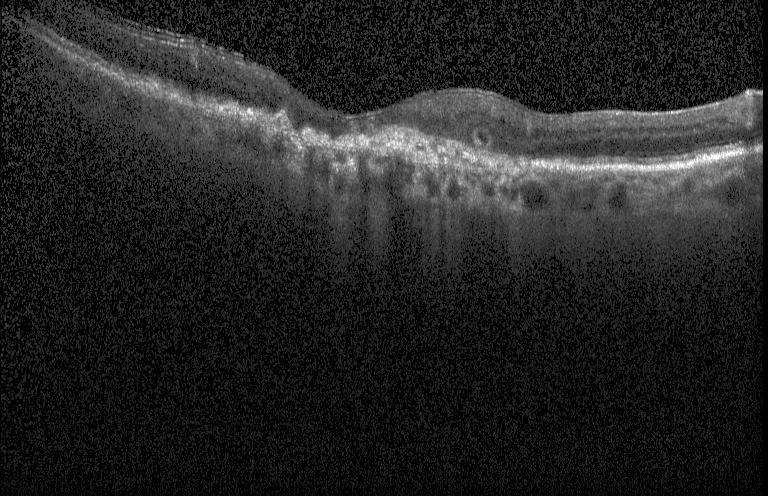
OCT B-scan, Heidelberg Spectralis OCT system, SD-OCT
Diagnosis: choroidal neovascularization.